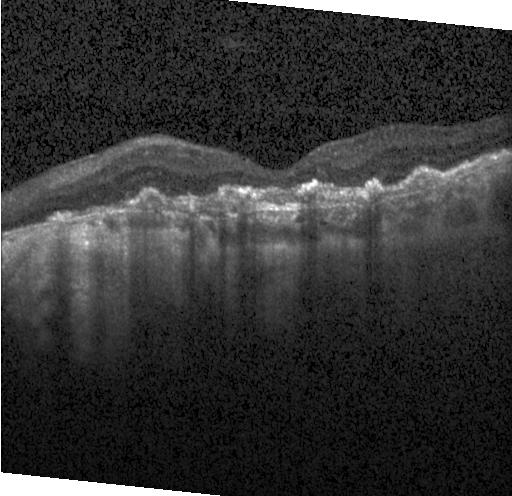 Dx: choroidal neovascularization.